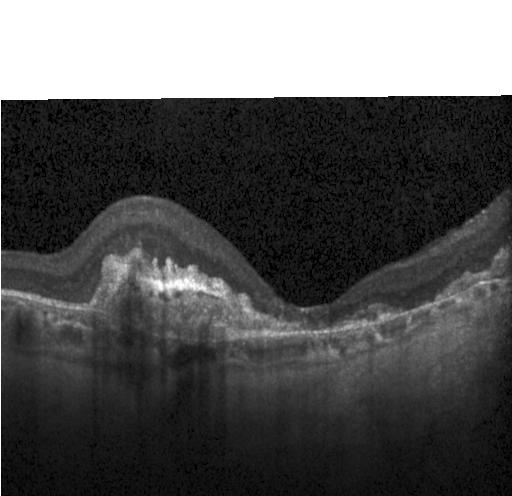 Horizontal scan through the fovea, optical coherence tomography scan, spectral-domain OCT, Heidelberg Spectralis OCT system — Diagnosis: a choroidal neovascular membrane.